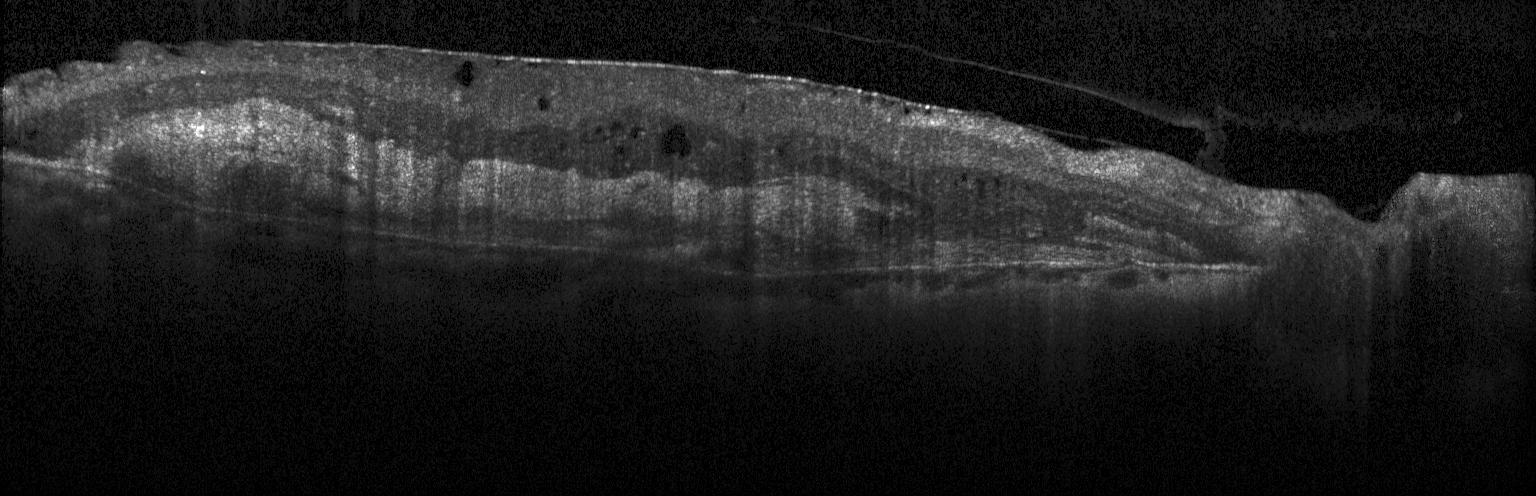

Optical coherence tomography scan. Dx: choroidal neovascularization.